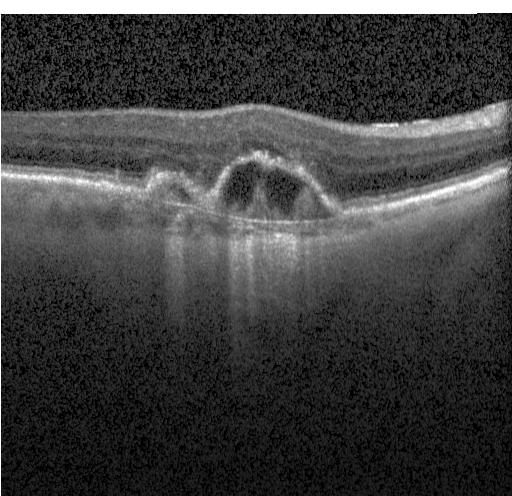

The scan shows a choroidal neovascular membrane.